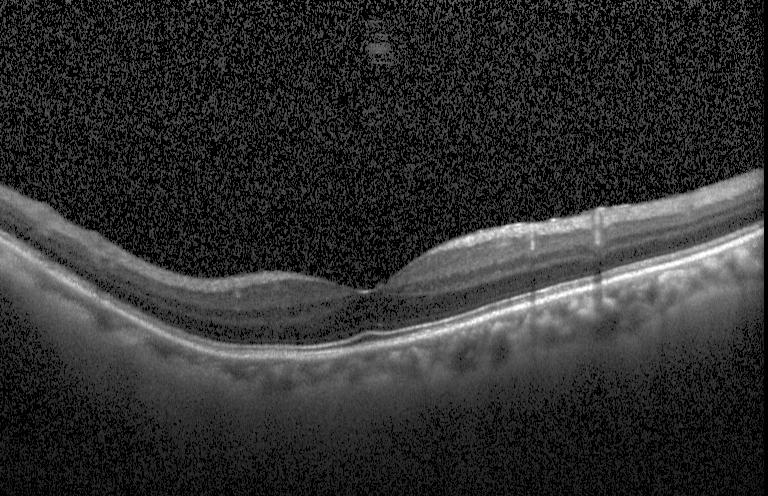
Diagnosis: no choroidal neovascularization, no diabetic macular edema, and no drusen.